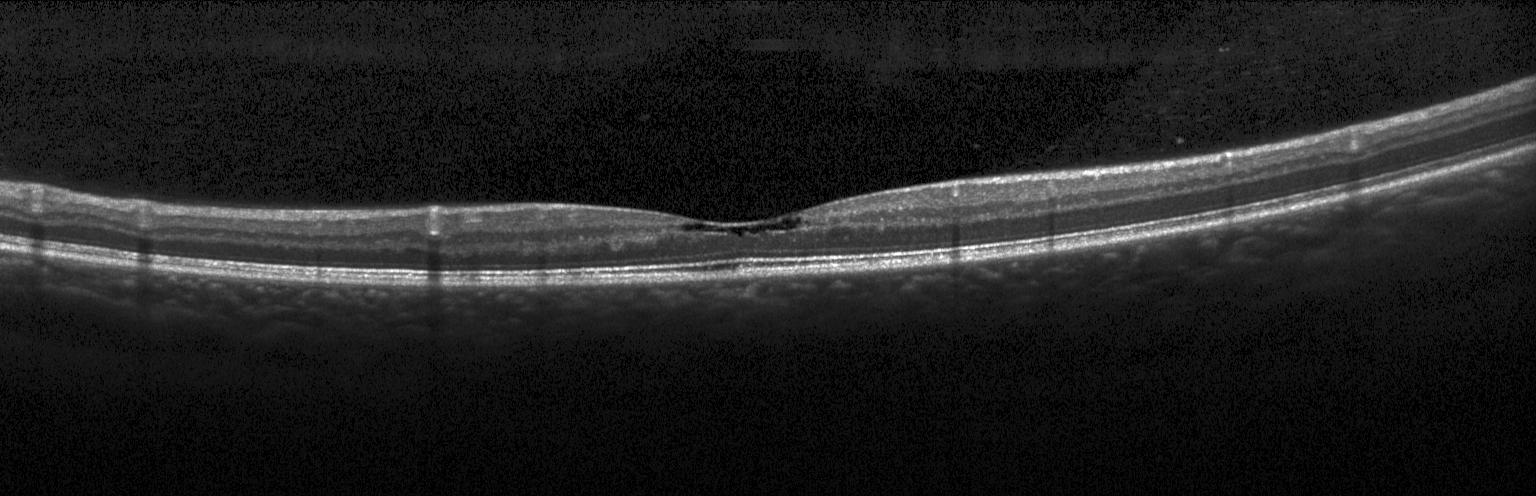

Horizontal scan through the fovea. Optical coherence tomography scan — Assessment: diabetic macular edema (DME).